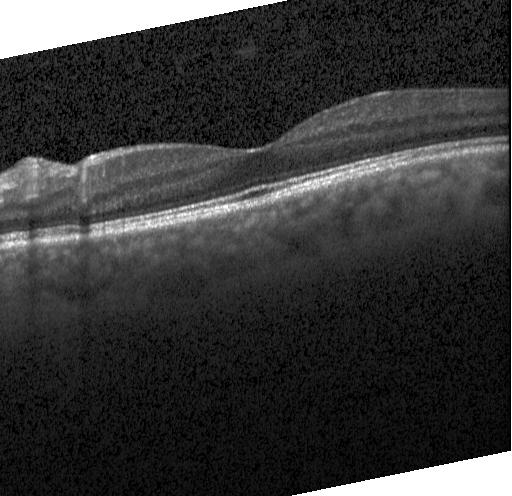 Retinal OCT cross-section.
Macular OCT: no choroidal neovascularization, no diabetic macular edema, and no drusen.